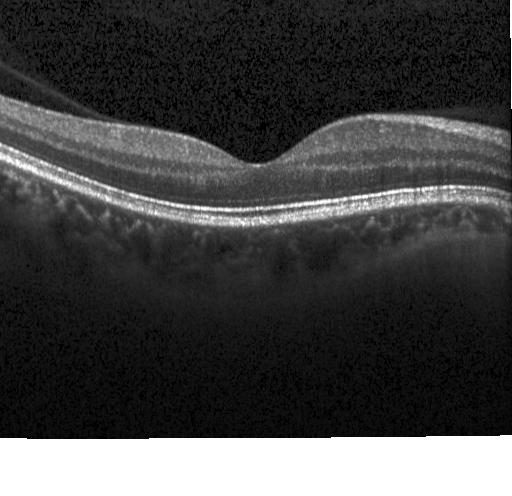 Instrument: Heidelberg Spectralis; retinal OCT B-scan; through the macula.
No choroidal neovascularization, diabetic macular edema, or drusen.